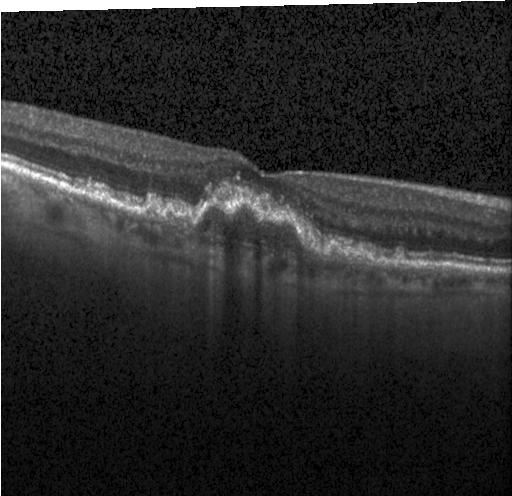

Retinal OCT cross-section · Heidelberg Spectralis OCT system · through the macula.
The scan shows choroidal neovascularization.